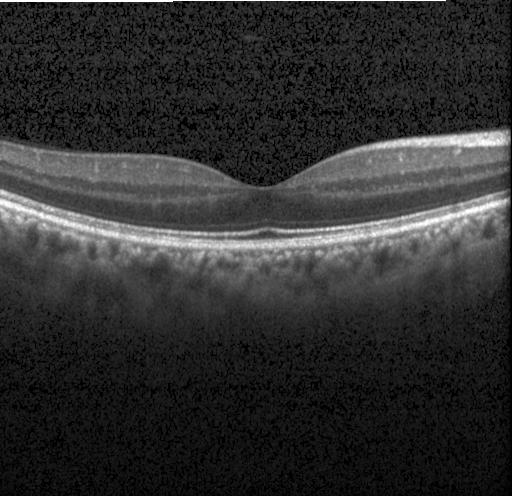

Through the macula, spectral-domain OCT, retinal OCT B-scan, acquired on a Heidelberg Spectralis. Assessment: neither choroidal neovascularization, diabetic macular edema, nor drusen.